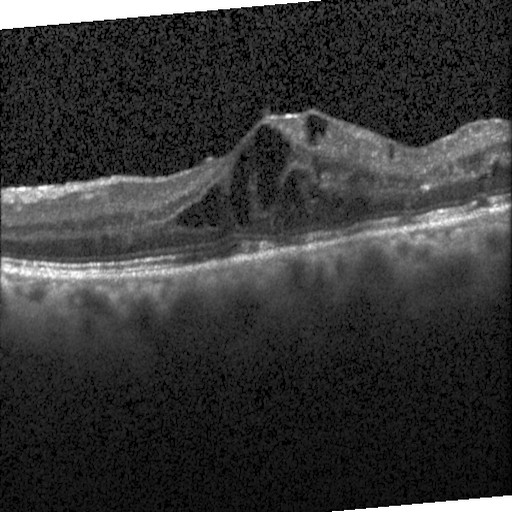
Horizontal scan through the fovea, optical coherence tomography B-scan, SD-OCT. Diagnosis: diabetic macular edema.